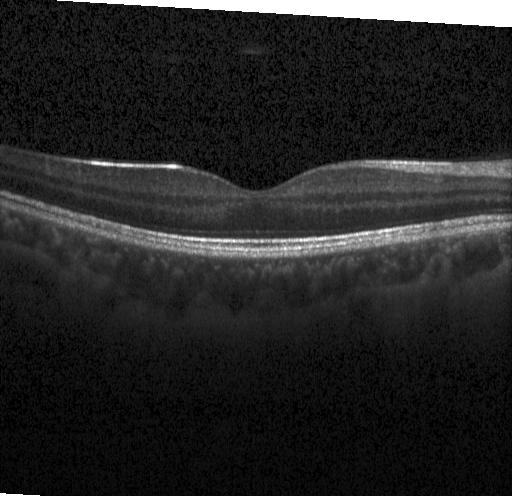

SD-OCT. OCT B-scan. Centered on the fovea — Impression: no evidence of CNV, DME, or drusen.